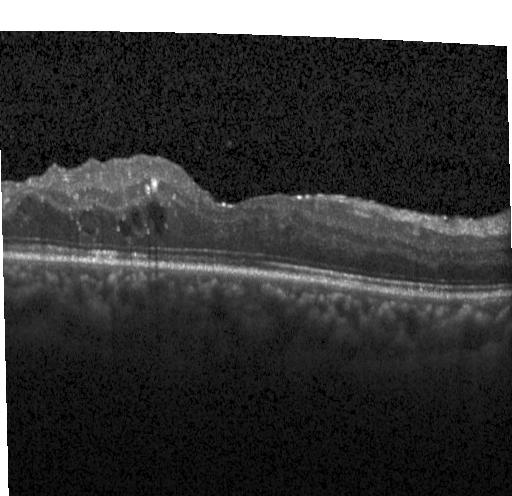
Retinal OCT cross-section — This B-scan demonstrates diabetic macular edema (DME).